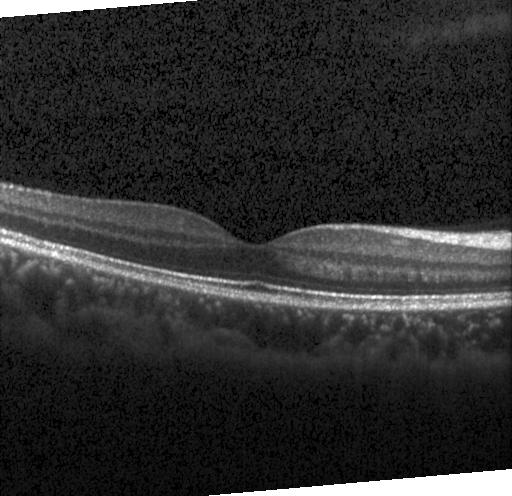

OCT B-scan; fovea-centered
This B-scan demonstrates no choroidal neovascularization, no diabetic macular edema, and no drusen.